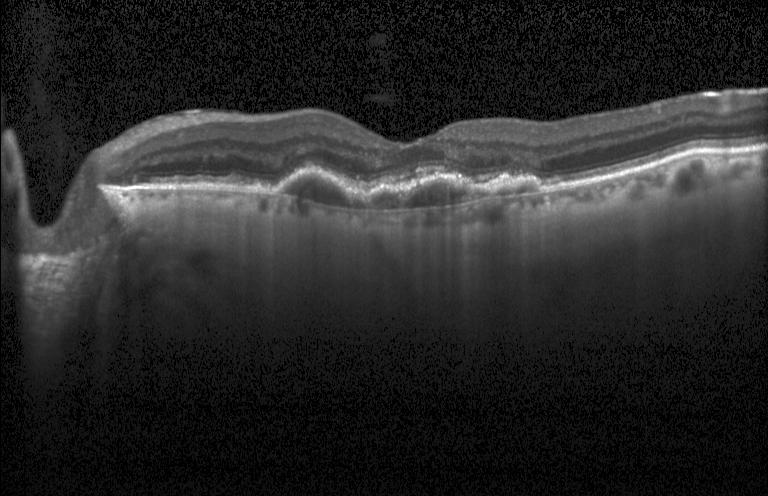
Heidelberg Spectralis · fovea-centered · SD-OCT · OCT B-scan
A choroidal neovascular membrane.